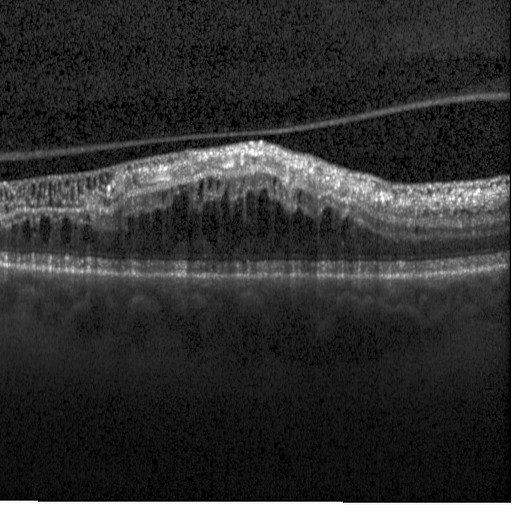
DME.